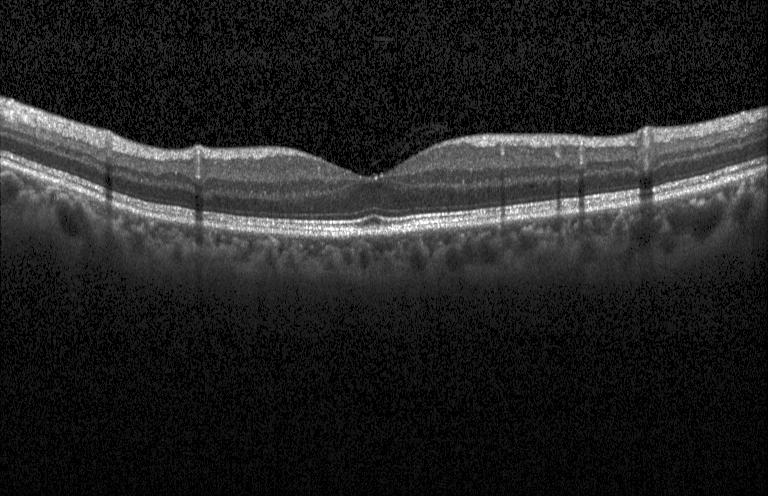

Heidelberg Spectralis OCT system. OCT B-scan
Neither choroidal neovascularization, diabetic macular edema, nor drusen.